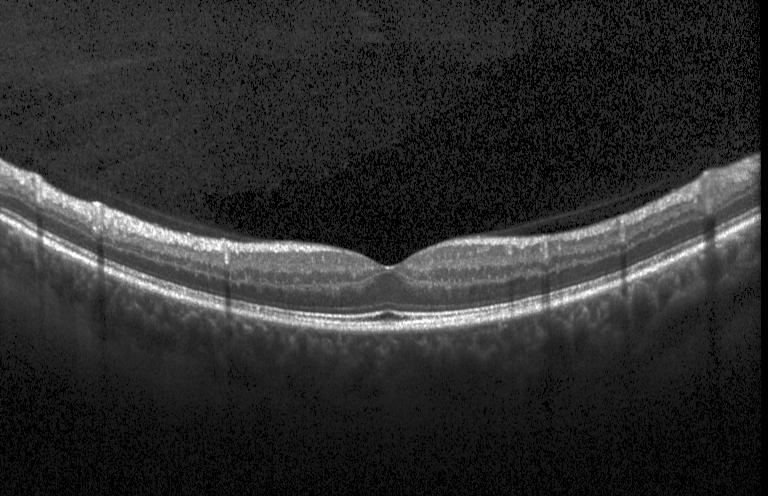 Fovea-centered. Spectral-domain optical coherence tomography. Heidelberg Spectralis. Optical coherence tomography B-scan.
OCT finding: neither choroidal neovascularization, diabetic macular edema, nor drusen.